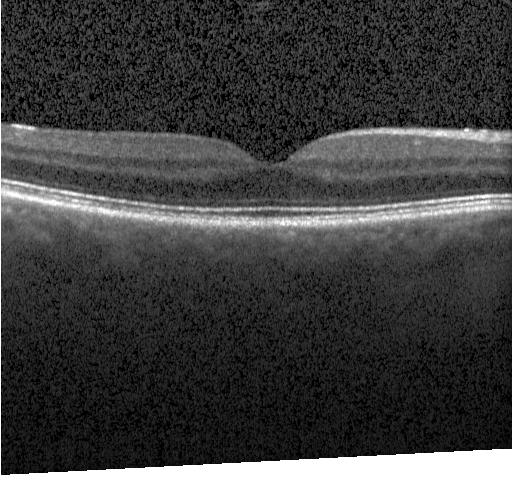

SD-OCT. Optical coherence tomography scan. Fovea-centered.
The scan shows no choroidal neovascularization, no diabetic macular edema, and no drusen.